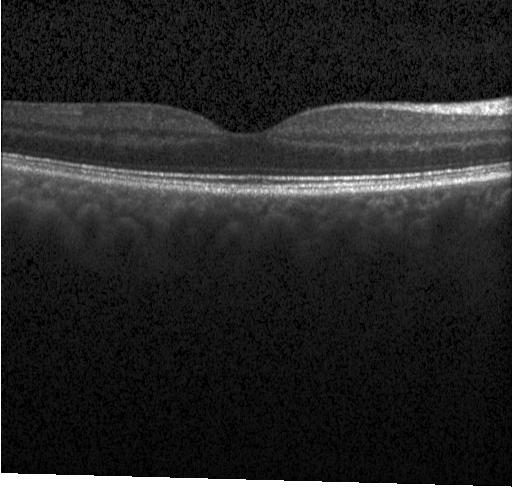

Finding: neither choroidal neovascularization, diabetic macular edema, nor drusen.